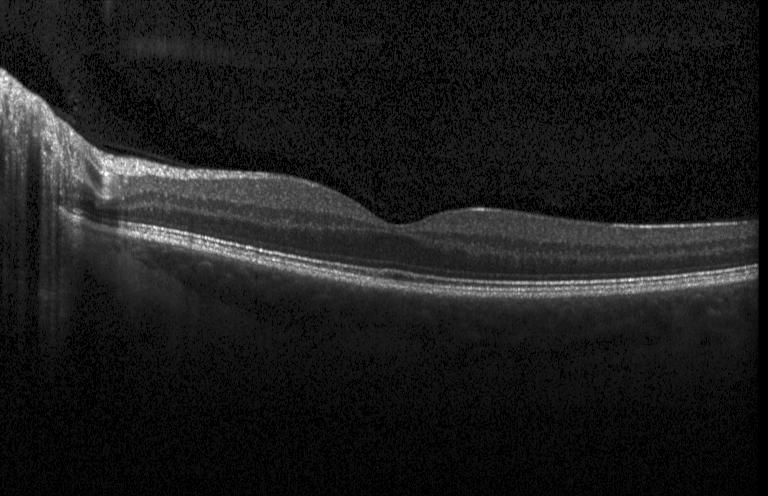

OCT B-scan; through the macula; spectral-domain optical coherence tomography.
Impression: no choroidal neovascularization, diabetic macular edema, or drusen.